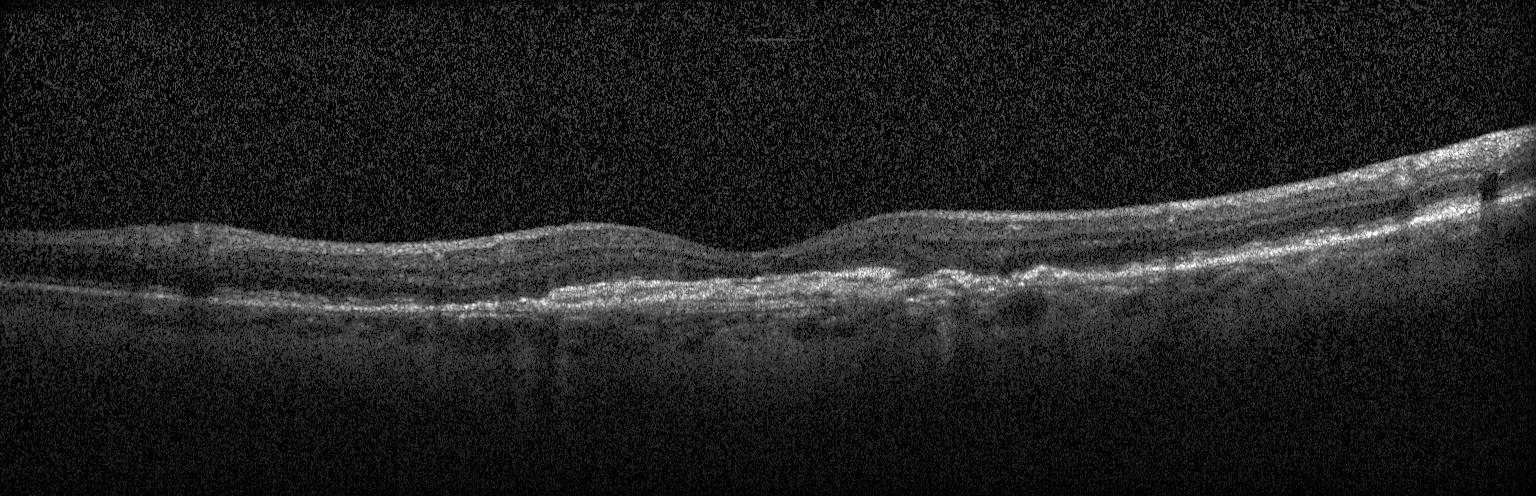 Retinal OCT B-scan, instrument: Heidelberg Spectralis — Diagnosis: CNV.